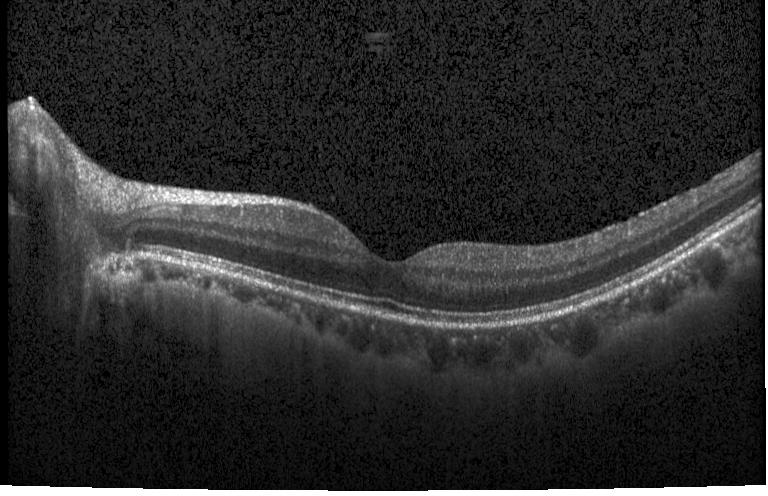
OCT B-scan, through the macula. Diagnosis: neither CNV, DME, nor drusen.